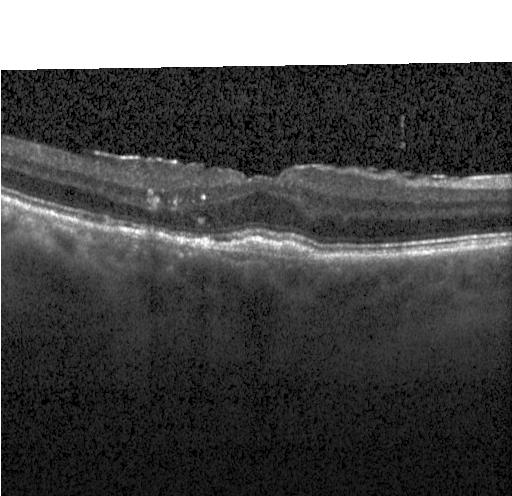

OCT finding: a choroidal neovascular membrane.